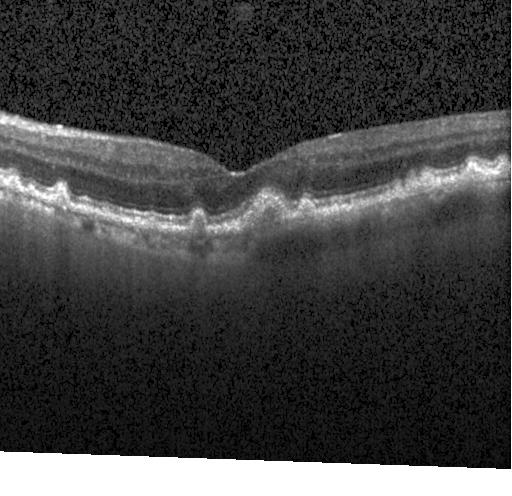
OCT scan showing multiple drusen.